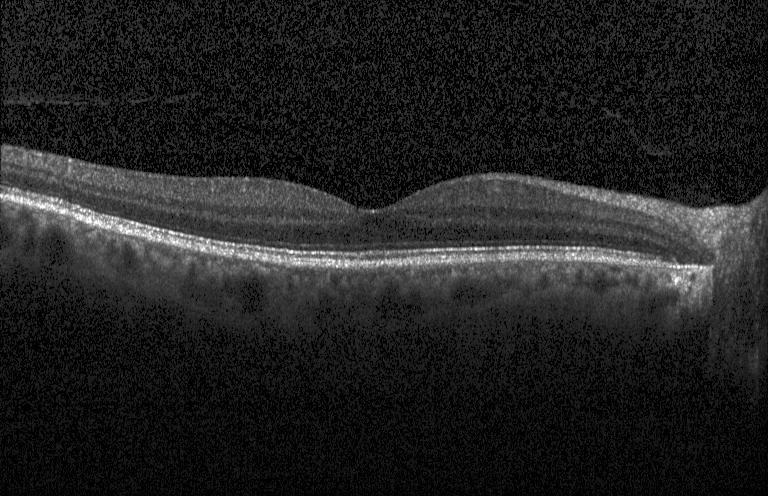 Optical coherence tomography B-scan · Heidelberg Spectralis OCT system. Assessment: no CNV, no DME, and no drusen.